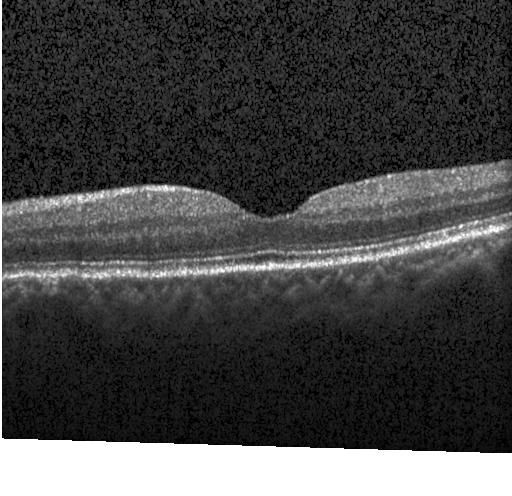

OCT line scan
Finding: neither choroidal neovascularization, diabetic macular edema, nor drusen.